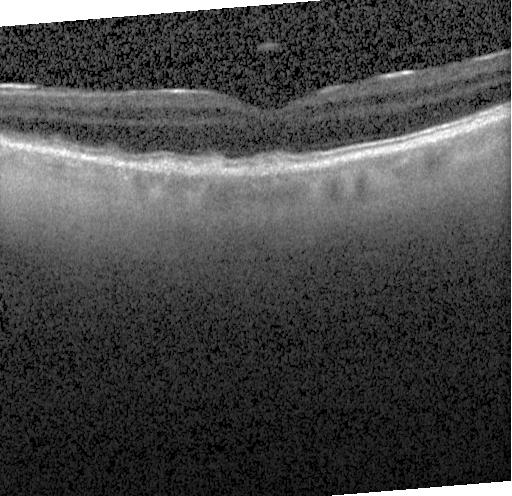
OCT B-scan. Macular scan.
Macular OCT: multiple drusen.